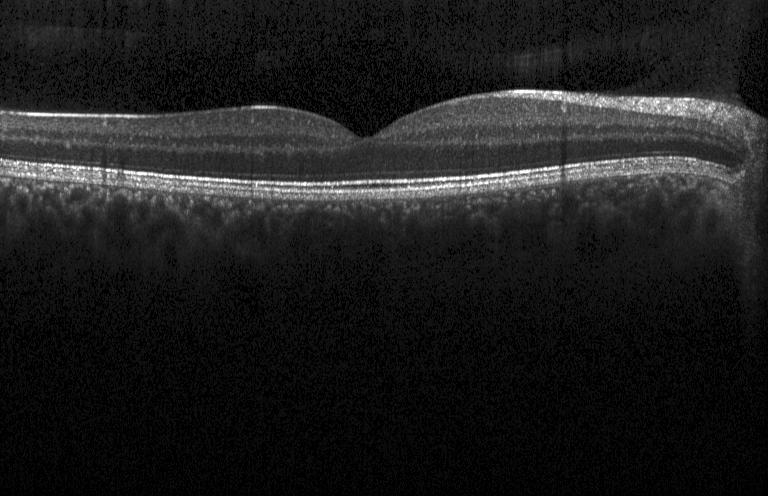

Spectral-domain OCT B-scan: neither choroidal neovascularization, diabetic macular edema, nor drusen.